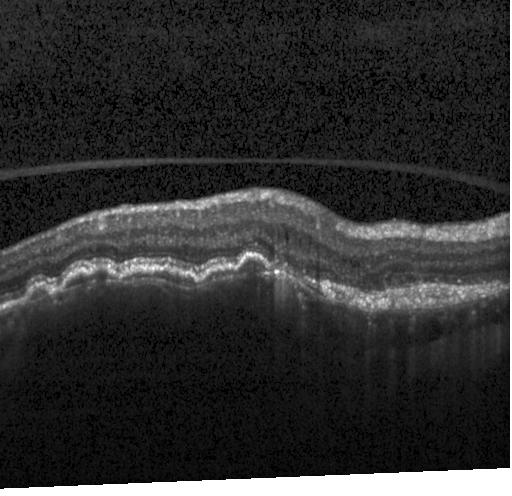
Impression: CNV.